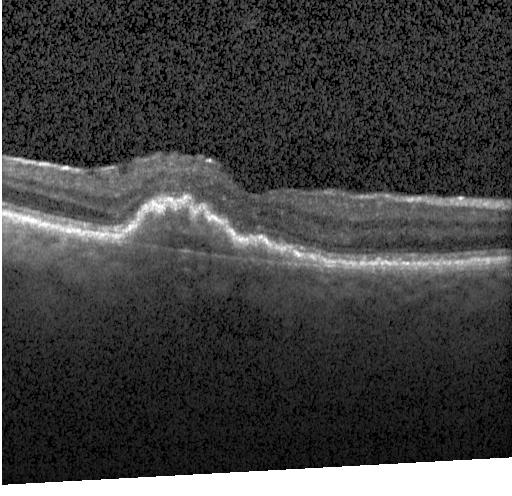
Spectral-domain OCT; macular scan; optical coherence tomography B-scan — Finding: choroidal neovascularization (CNV).